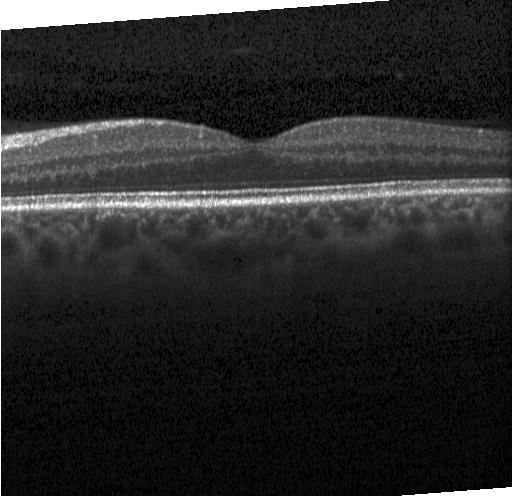

Retinal OCT cross-section showing neither choroidal neovascularization, diabetic macular edema, nor drusen.